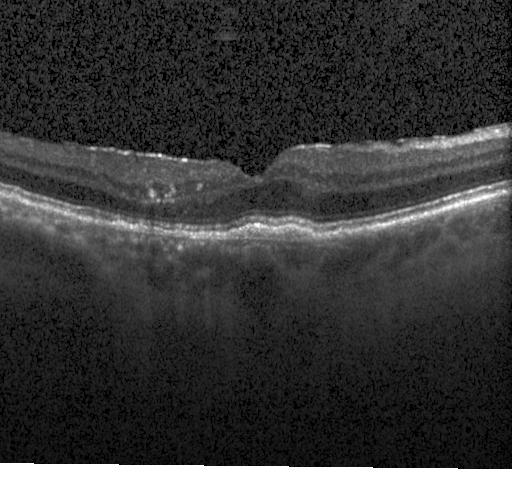
Centered on the fovea. Optical coherence tomography B-scan — This B-scan demonstrates choroidal neovascularization.